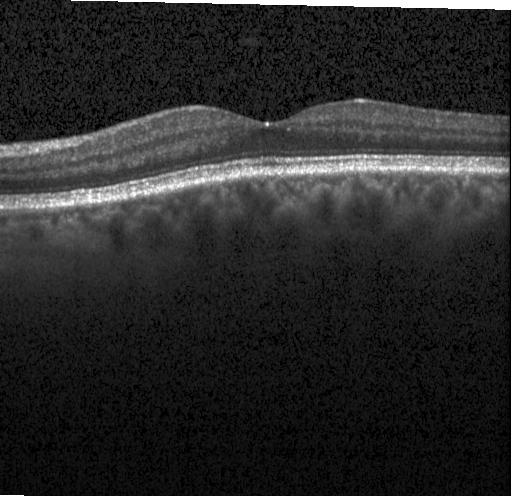
Finding: neither choroidal neovascularization, diabetic macular edema, nor drusen.